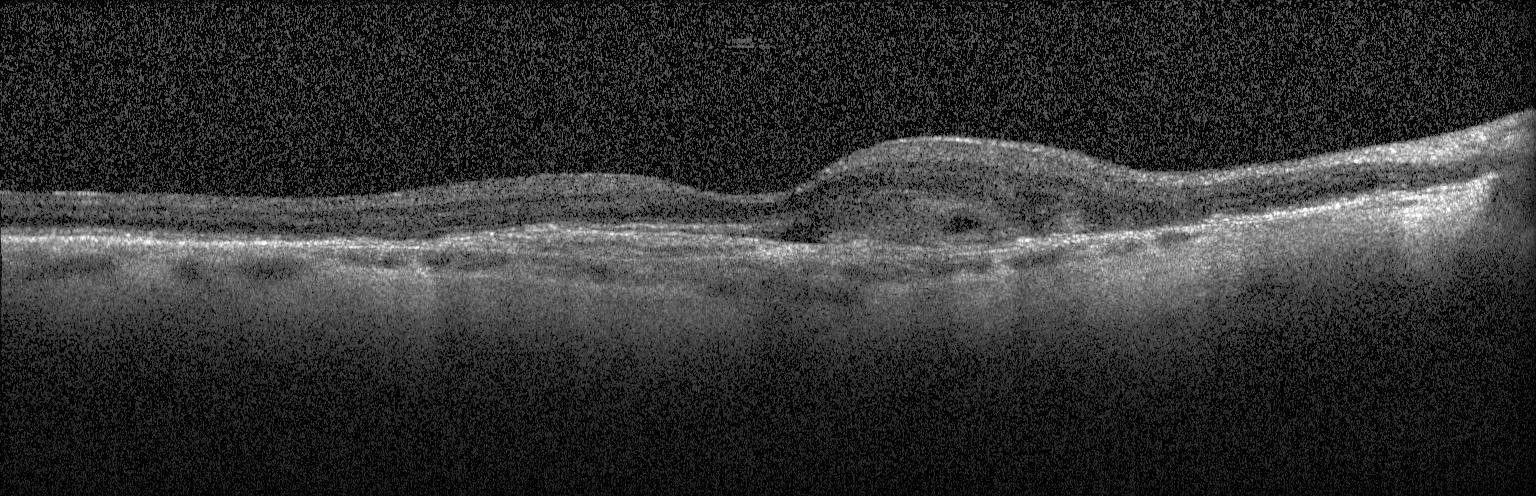 Heidelberg Spectralis. Retinal OCT cross-section. Diagnosis: CNV.